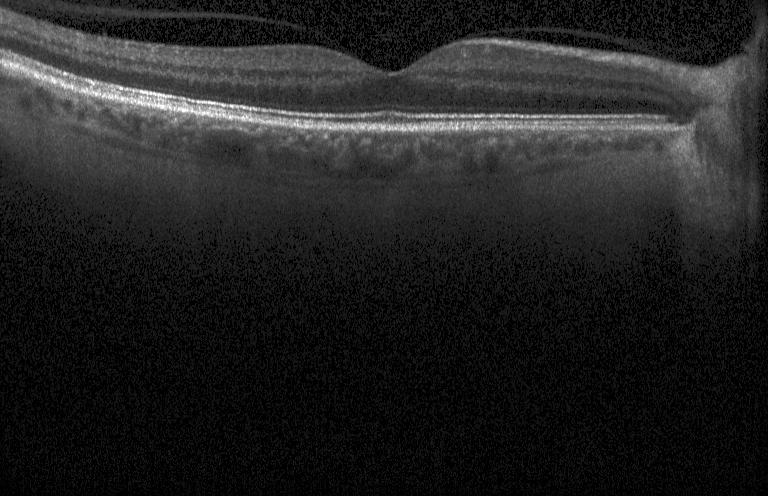
OCT B-scan
Assessment: no choroidal neovascularization, no diabetic macular edema, and no drusen.